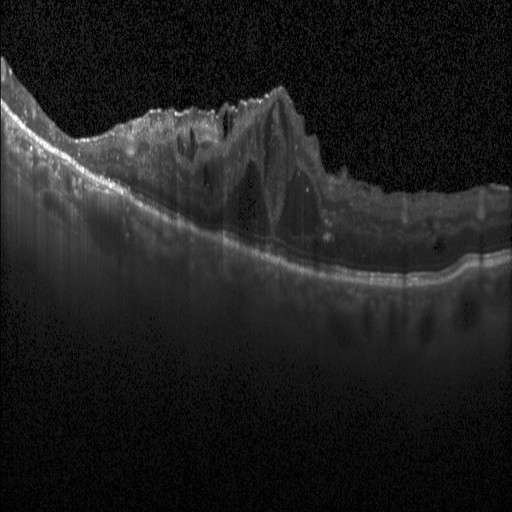 Spectral-domain optical coherence tomography; Heidelberg Spectralis; macular scan; retinal OCT cross-section.
This B-scan demonstrates DME.